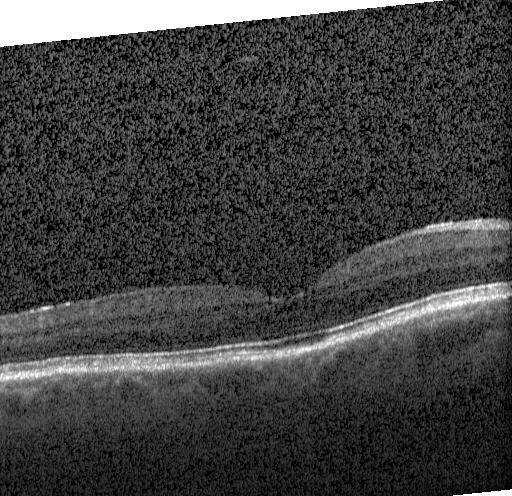
Optical coherence tomography scan. OCT finding: neither CNV, DME, nor drusen.